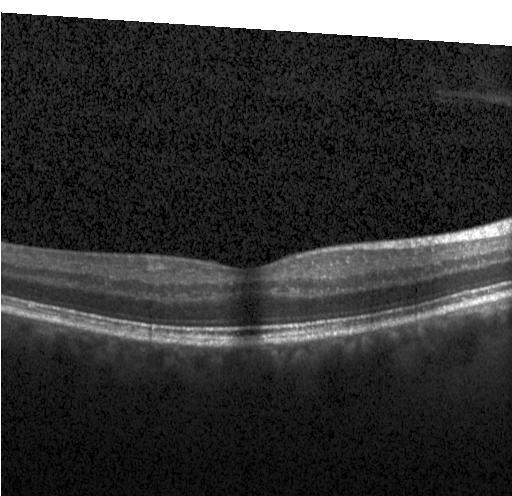
Heidelberg Spectralis. Retinal OCT B-scan. Through the macula. Spectral-domain optical coherence tomography. Impression: no choroidal neovascularization, no diabetic macular edema, and no drusen.